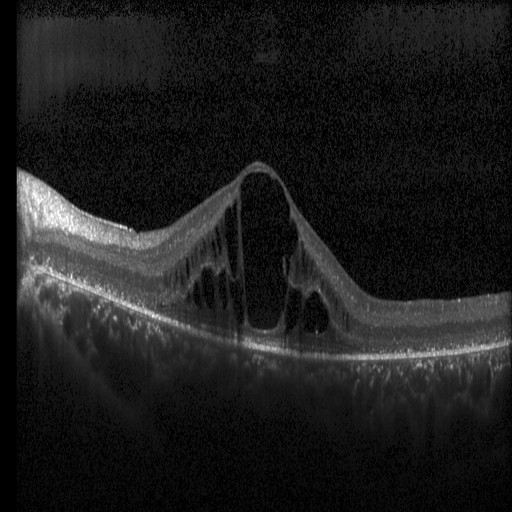
OCT B-scan. Diagnosis: diabetic macular edema.